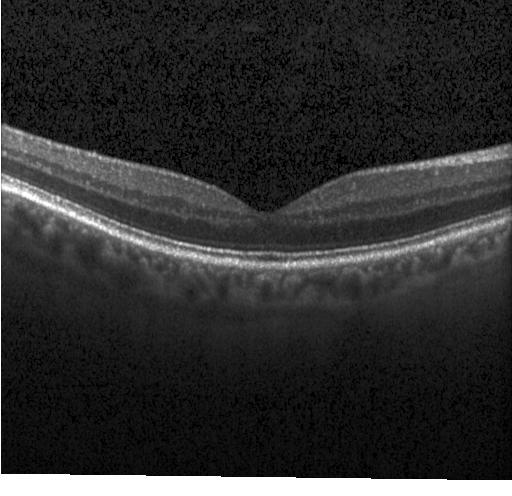

Diagnosis: no choroidal neovascularization, no diabetic macular edema, and no drusen.